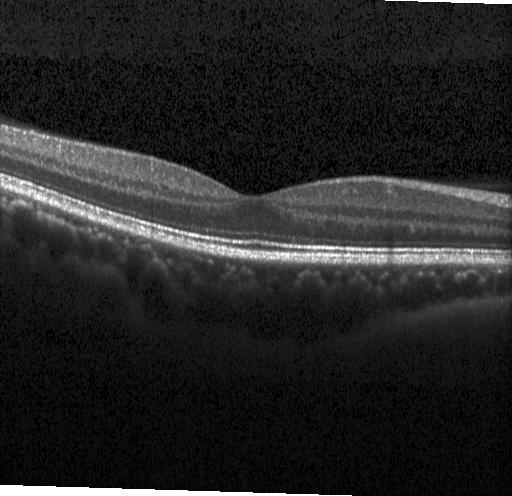 Retinal OCT cross-section, through the macula, Heidelberg Spectralis OCT system, spectral-domain OCT
No evidence of choroidal neovascularization, diabetic macular edema, or drusen.